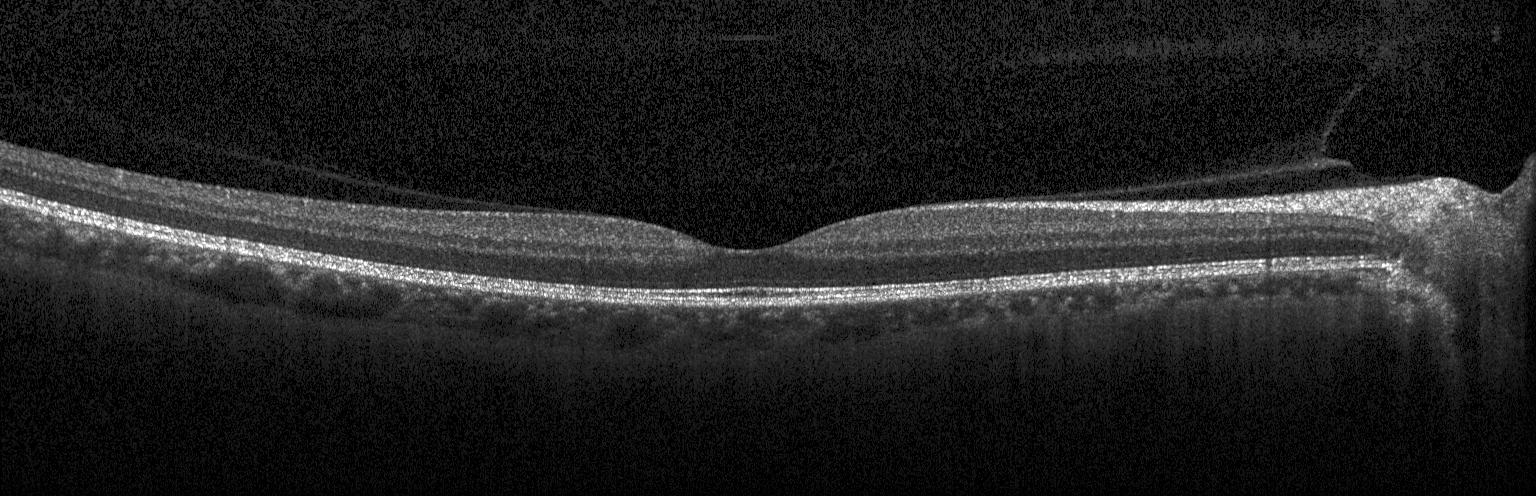 Spectral-domain optical coherence tomography, retinal OCT cross-section, Heidelberg Spectralis OCT system
This B-scan demonstrates no CNV, no DME, and no drusen.